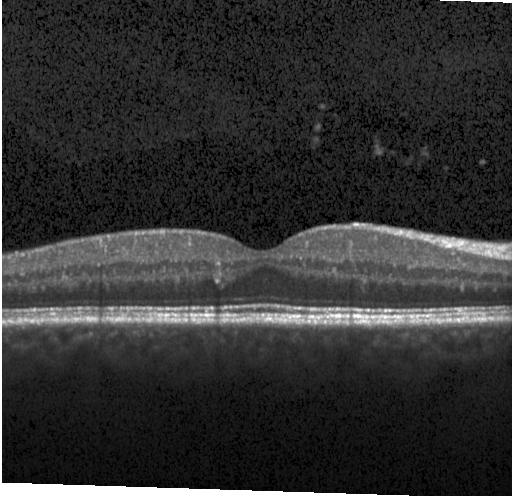
Dx: no evidence of choroidal neovascularization, diabetic macular edema, or drusen.